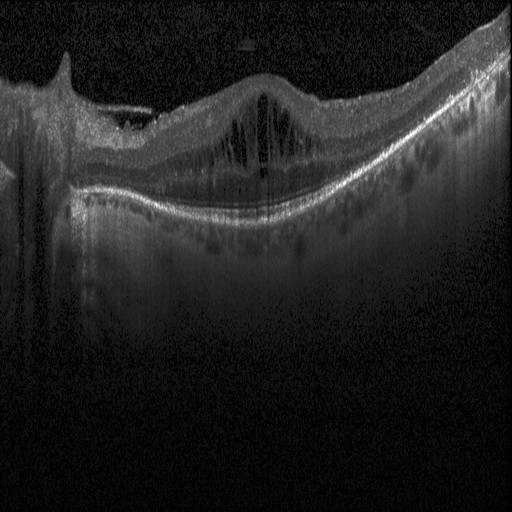

Finding: DME.